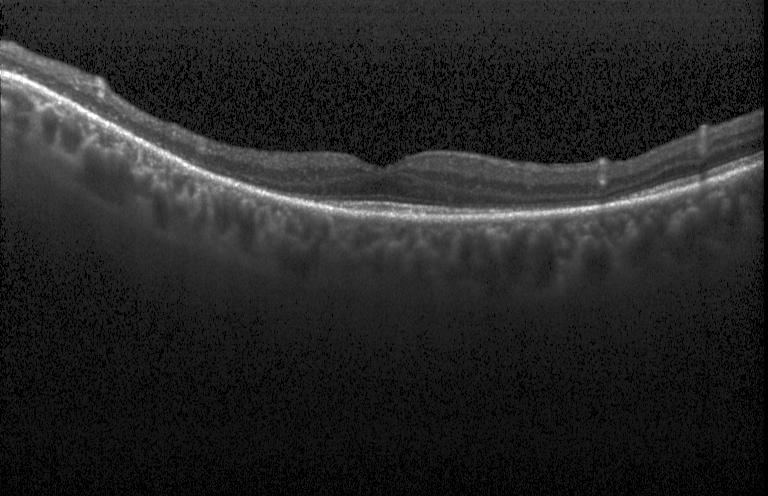 Diagnosis: no choroidal neovascularization, diabetic macular edema, or drusen.